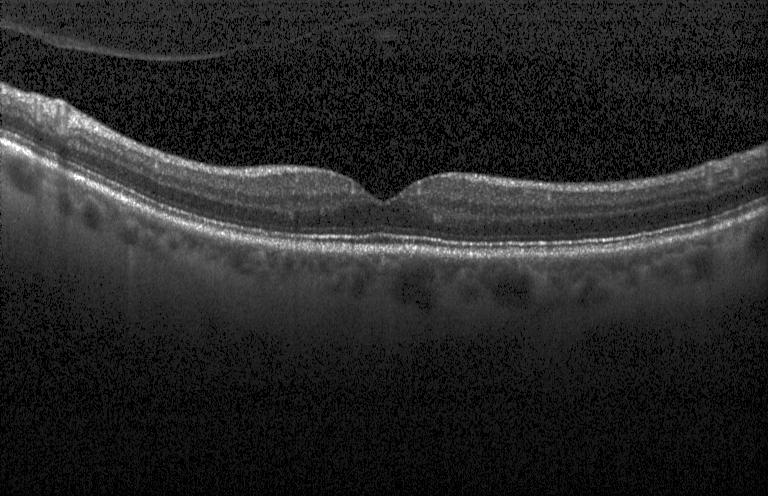

Optical coherence tomography B-scan — Finding: neither choroidal neovascularization, diabetic macular edema, nor drusen.